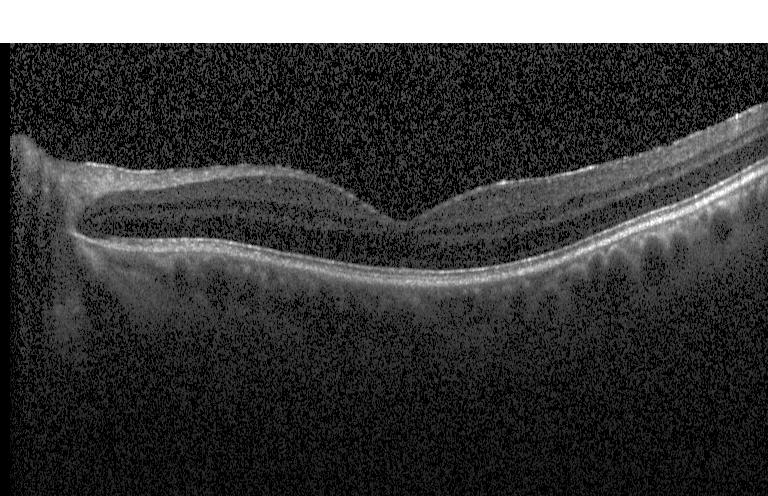
Impression: no evidence of choroidal neovascularization, diabetic macular edema, or drusen.